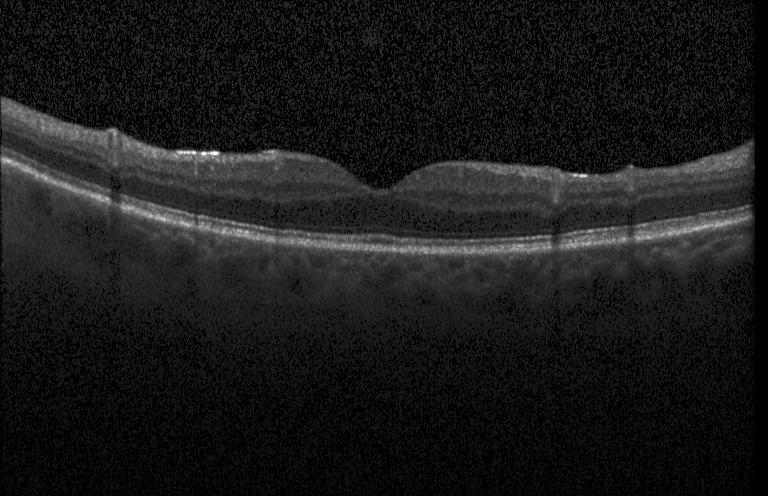 Retinal OCT B-scan.
Macular OCT: no CNV, DME, or drusen.